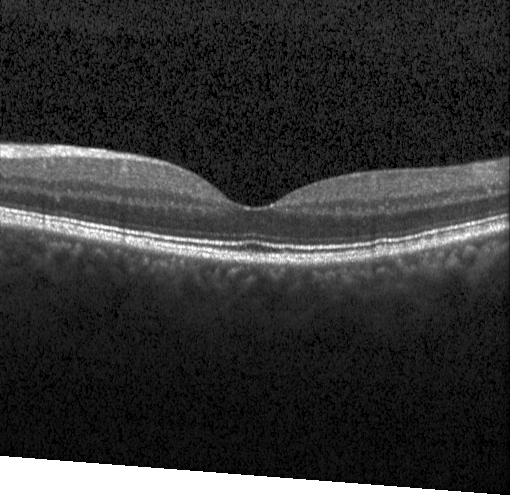
Horizontal scan through the fovea · retinal OCT B-scan — Impression: no choroidal neovascularization, no diabetic macular edema, and no drusen.